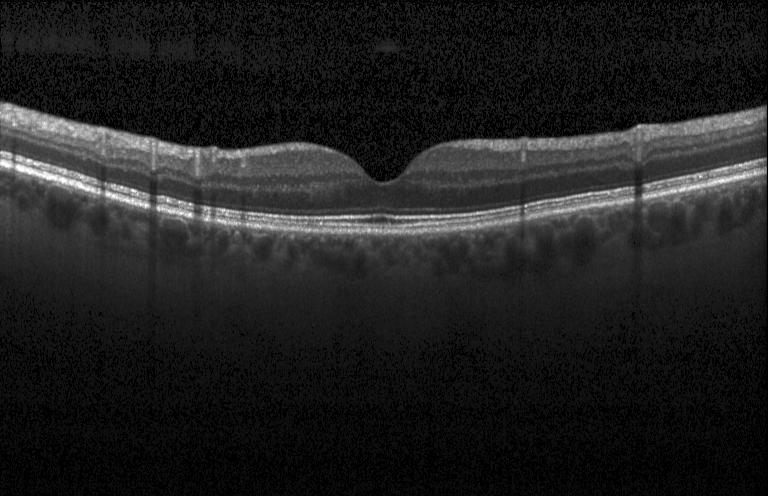 OCT finding: no evidence of choroidal neovascularization, diabetic macular edema, or drusen.